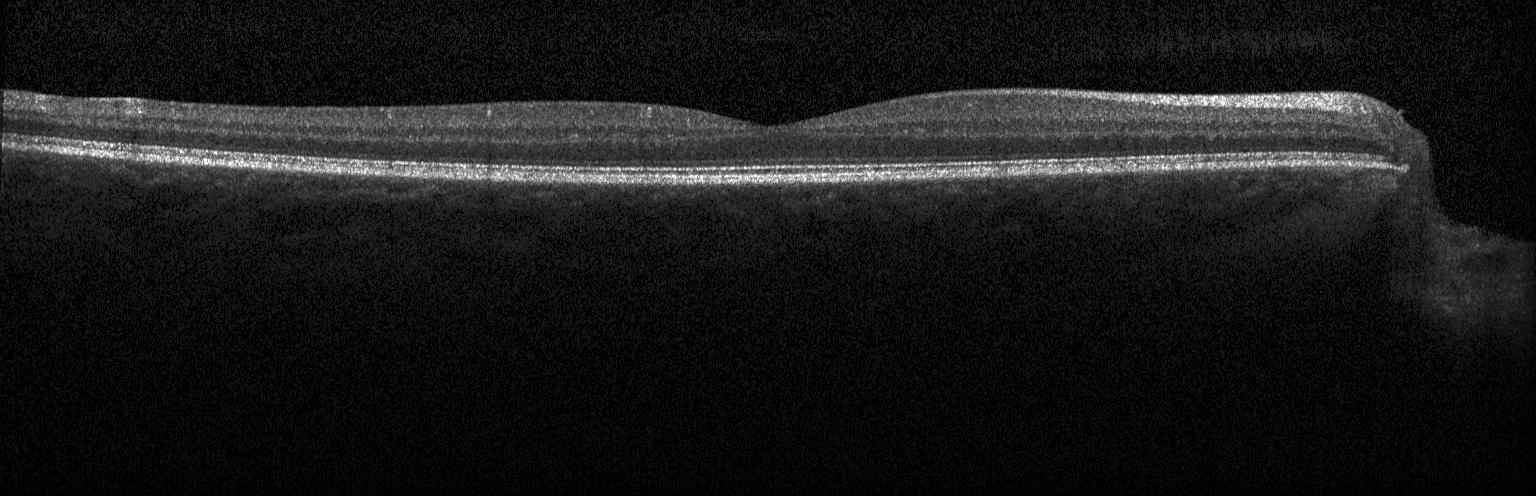 OCT line scan.
The scan shows no choroidal neovascularization, diabetic macular edema, or drusen.